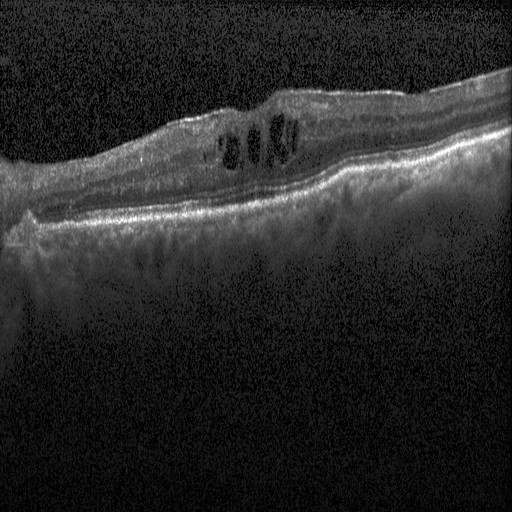
Spectral-domain OCT B-scan: diabetic macular edema (DME).